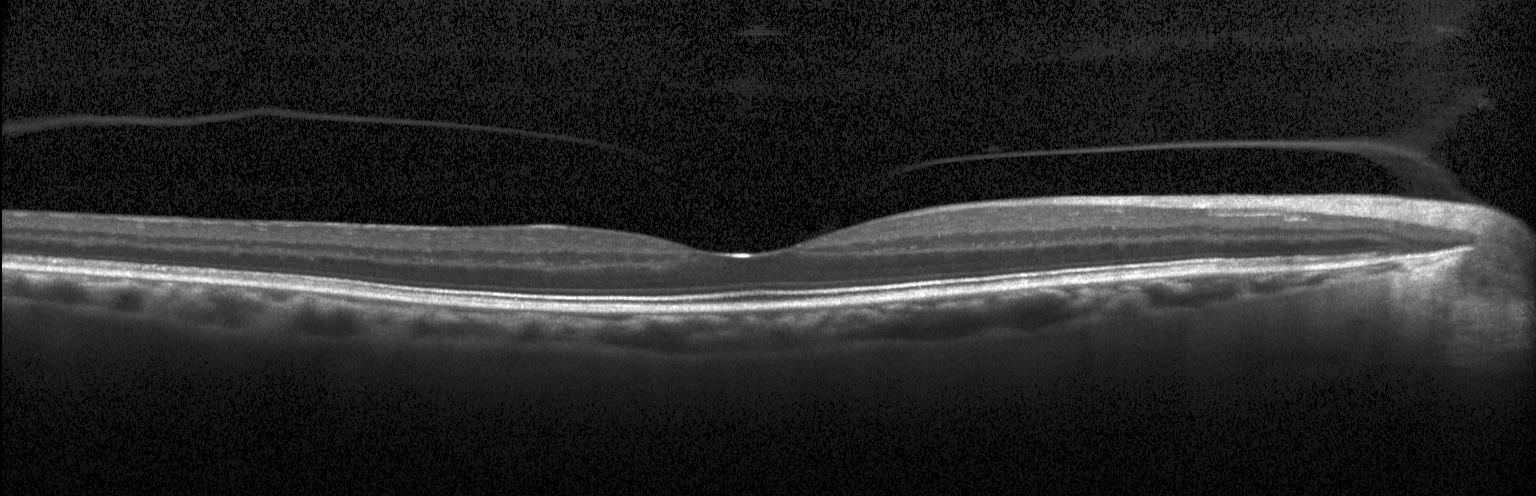 Macular OCT demonstrating neither choroidal neovascularization, diabetic macular edema, nor drusen.